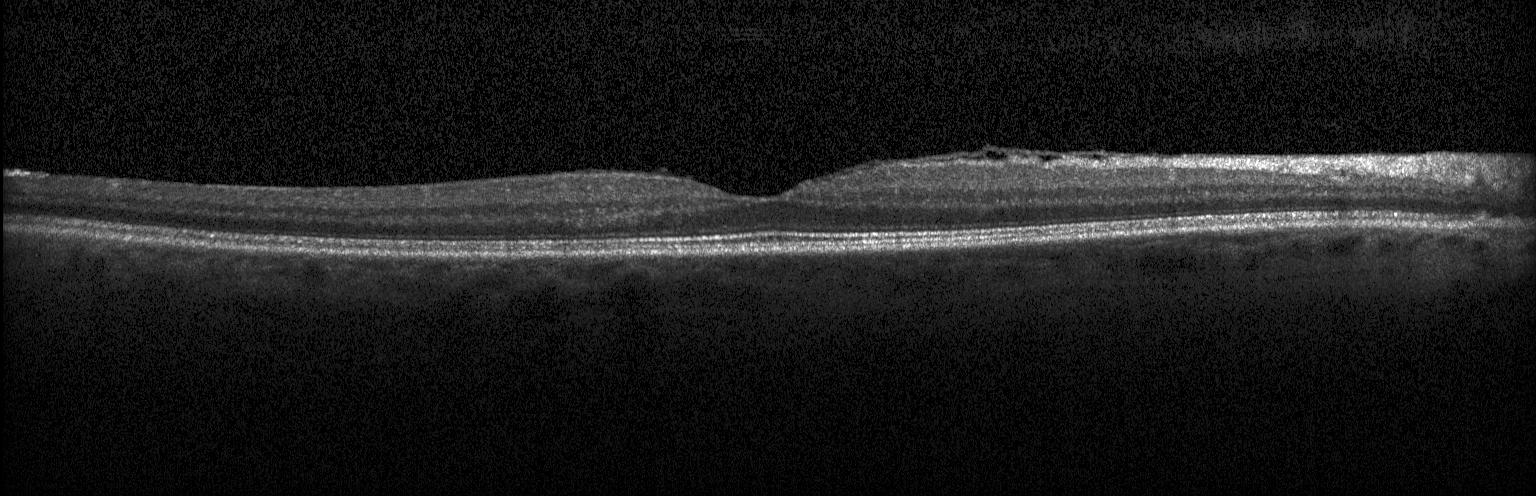
Optical coherence tomography scan; fovea-centered; Heidelberg Spectralis OCT system; spectral-domain optical coherence tomography — Diagnosis: neither choroidal neovascularization, diabetic macular edema, nor drusen.